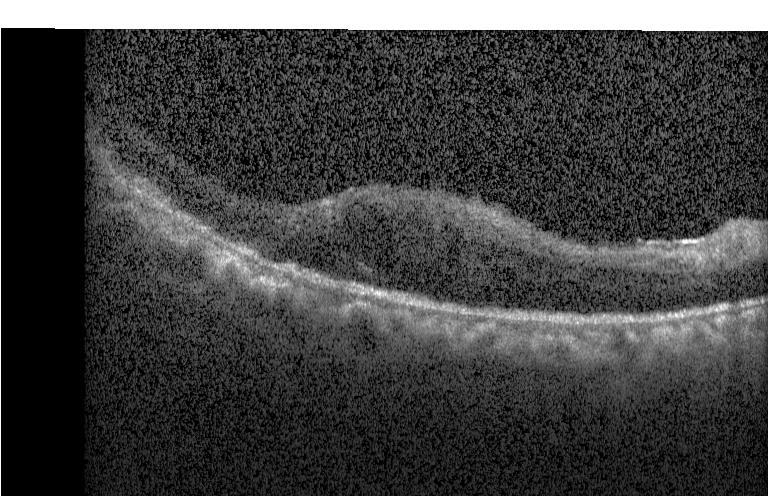

Impression: diabetic macular edema.